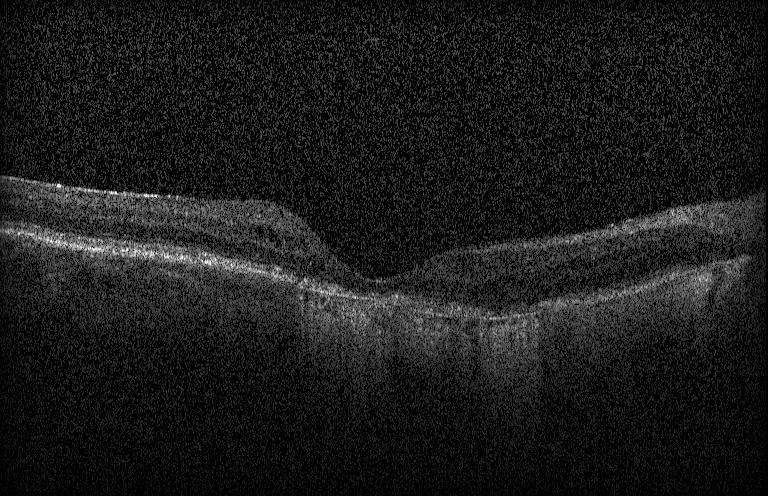

Impression: CNV.